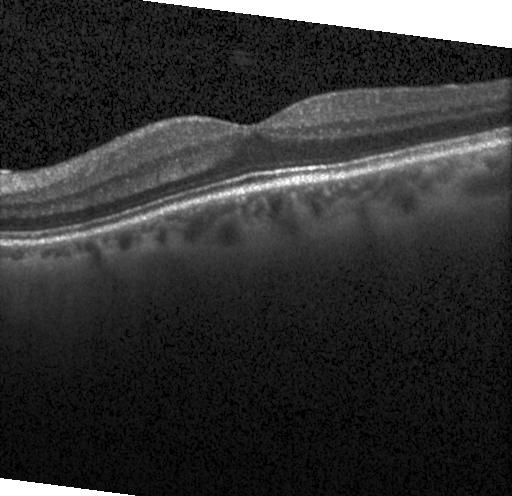

Macular scan, Heidelberg Spectralis OCT system, OCT B-scan — Macular OCT: no evidence of choroidal neovascularization, diabetic macular edema, or drusen.